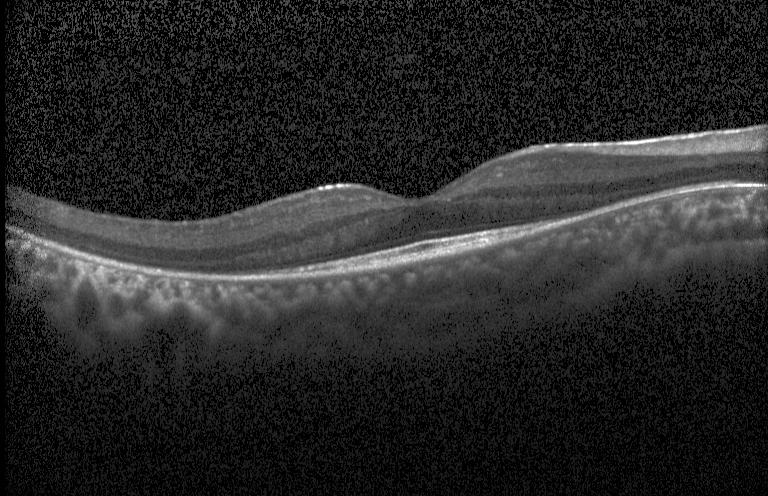 Assessment: no evidence of choroidal neovascularization, diabetic macular edema, or drusen.